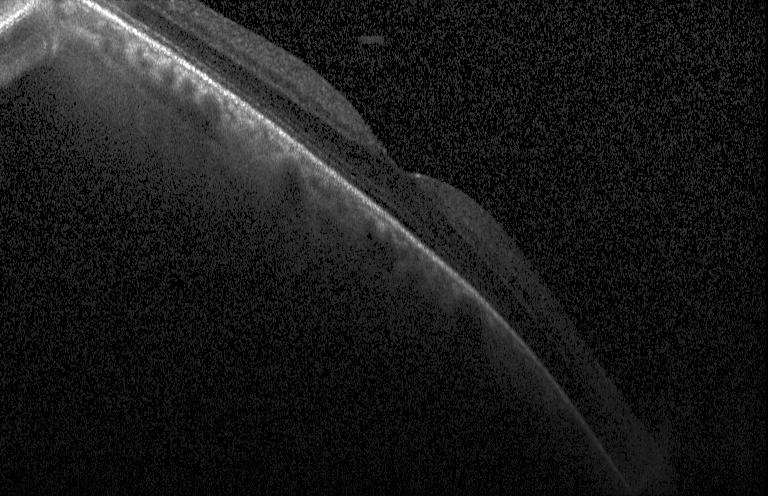 Instrument: Heidelberg Spectralis; retinal OCT cross-section; spectral-domain OCT; fovea-centered
OCT finding: no choroidal neovascularization, no diabetic macular edema, and no drusen.